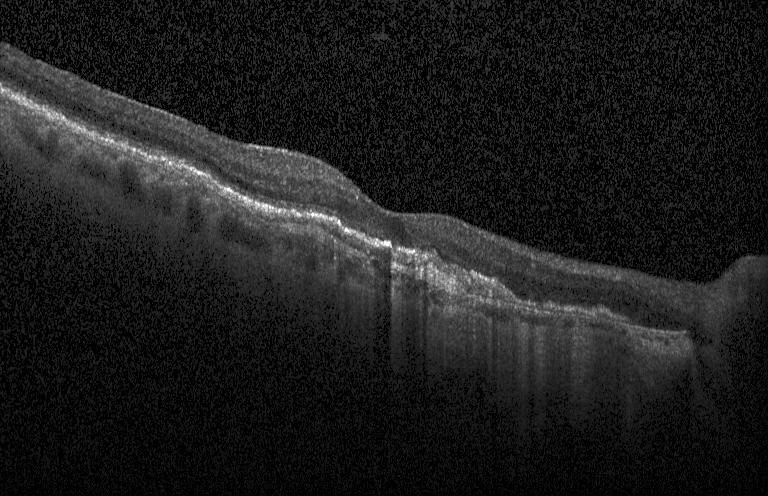

Horizontal scan through the fovea · spectral-domain optical coherence tomography · optical coherence tomography scan.
Diagnosis: CNV.